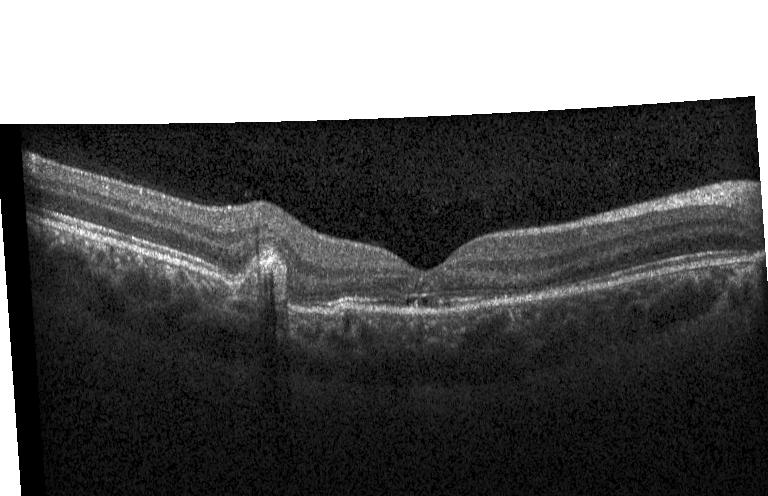 Retinal OCT B-scan.
Macular OCT: CNV.